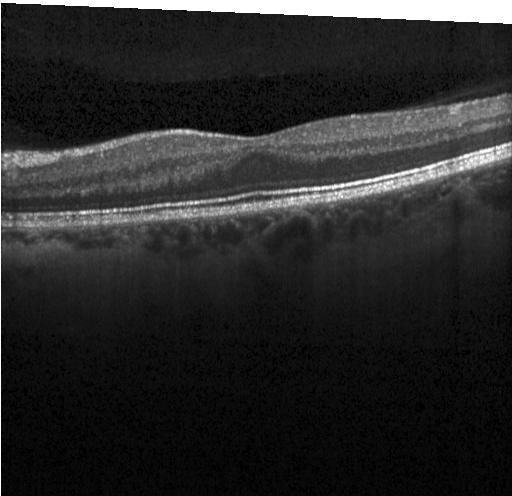
Horizontal scan through the fovea; OCT line scan.
Dx: no CNV, DME, or drusen.